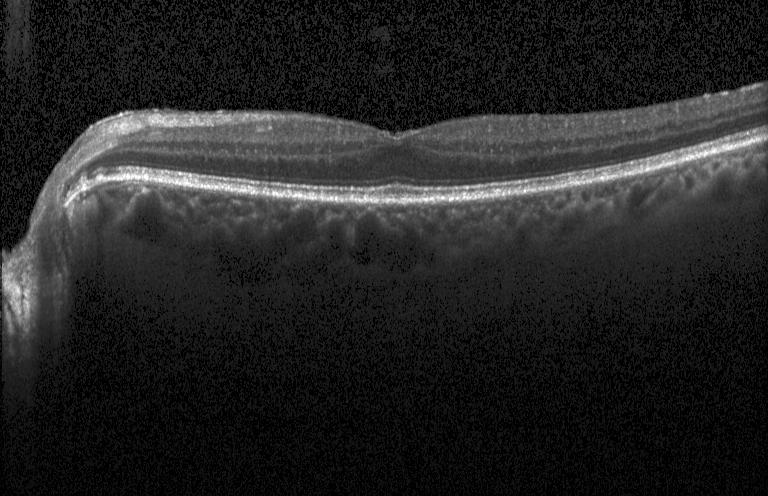 Spectral-domain optical coherence tomography · retinal OCT B-scan. Dx: neither choroidal neovascularization, diabetic macular edema, nor drusen.